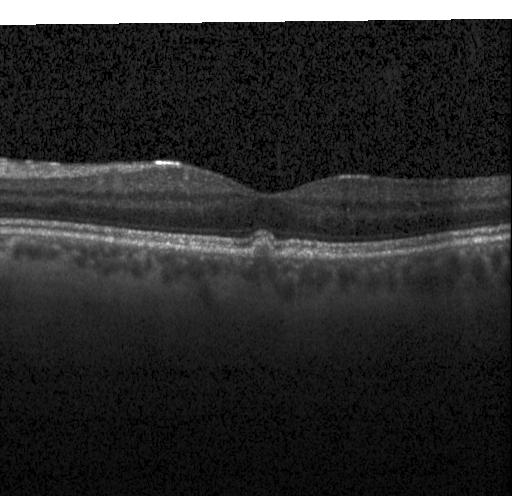 Spectral-domain optical coherence tomography. Optical coherence tomography B-scan.
Diagnosis: sub-RPE drusenoid deposits.